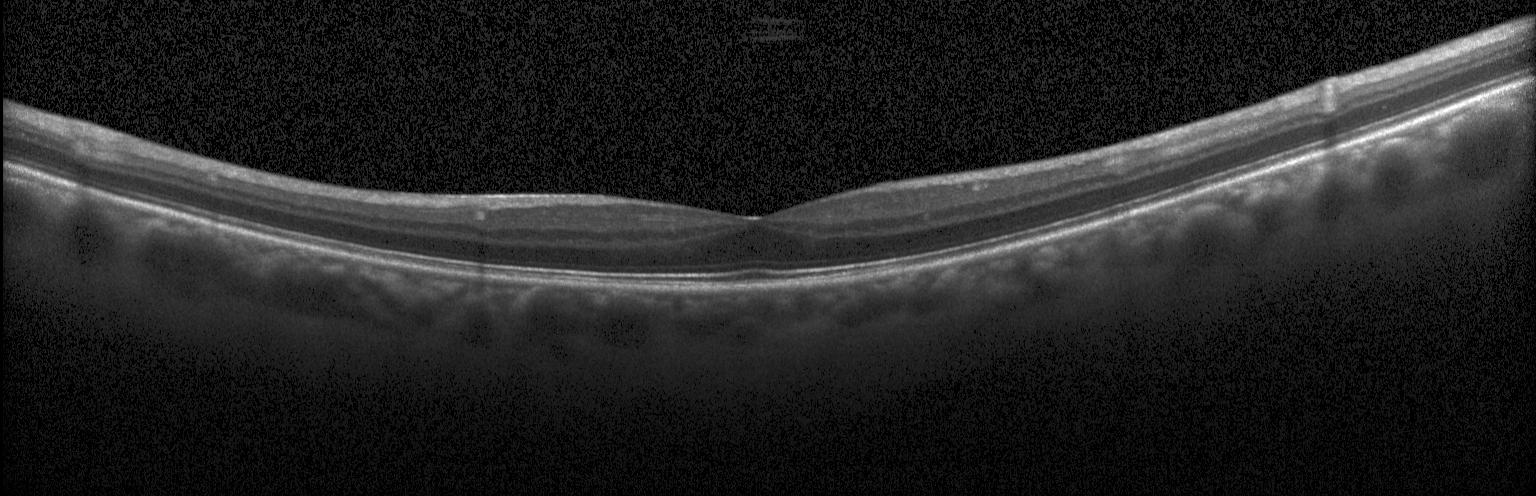
This B-scan demonstrates no choroidal neovascularization, no diabetic macular edema, and no drusen.